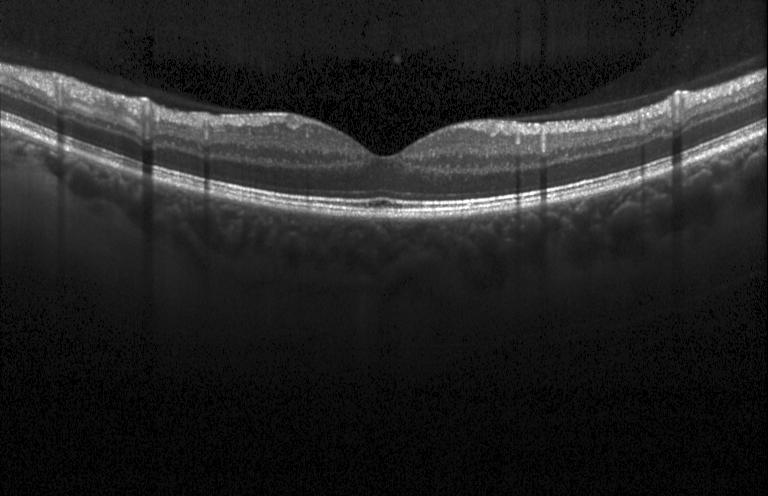 Spectral-domain optical coherence tomography. OCT line scan
Diagnosis: neither choroidal neovascularization, diabetic macular edema, nor drusen.